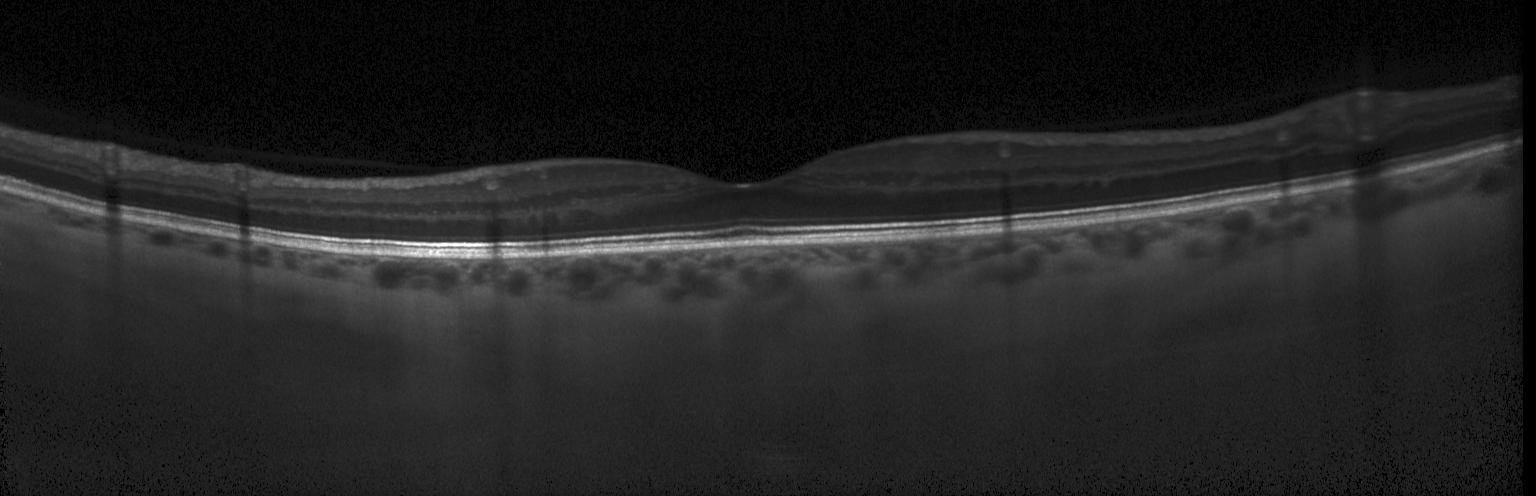 Assessment: no evidence of choroidal neovascularization, diabetic macular edema, or drusen.